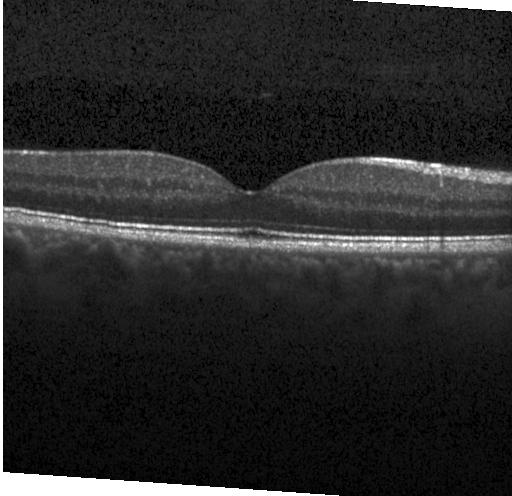
Instrument: Heidelberg Spectralis; OCT B-scan. This B-scan demonstrates no CNV, no DME, and no drusen.